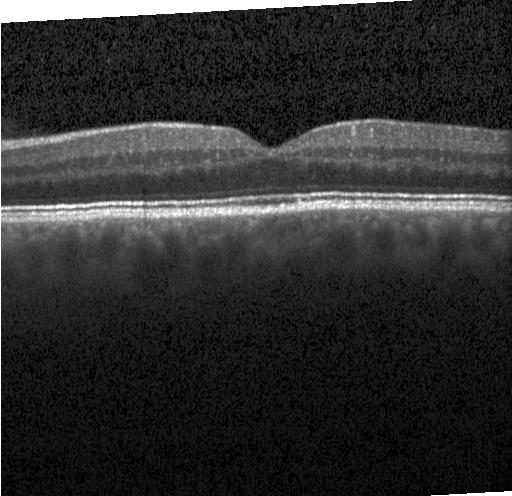

Diagnosis: no choroidal neovascularization, no diabetic macular edema, and no drusen.